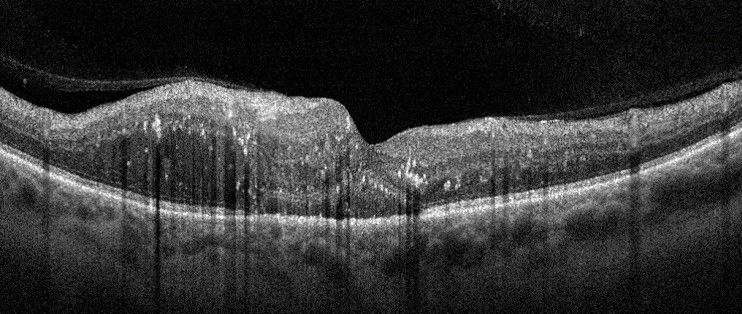 OCT line scan · instrument: Optovue Avanti RTVue XR · macular scan.
This B-scan demonstrates DME.